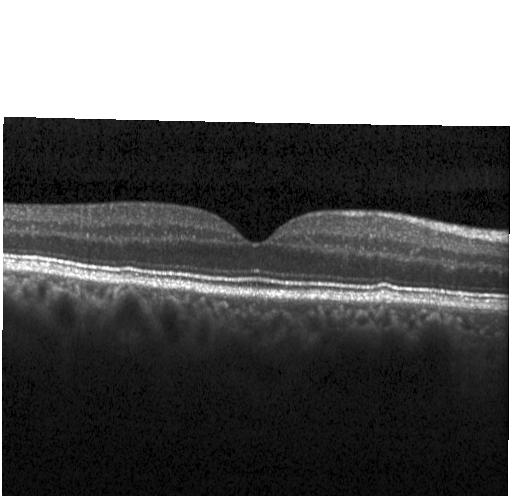

Finding: no evidence of choroidal neovascularization, diabetic macular edema, or drusen.